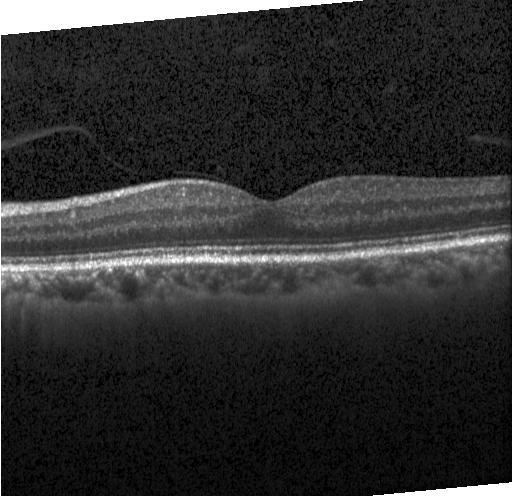 Dx: neither choroidal neovascularization, diabetic macular edema, nor drusen.